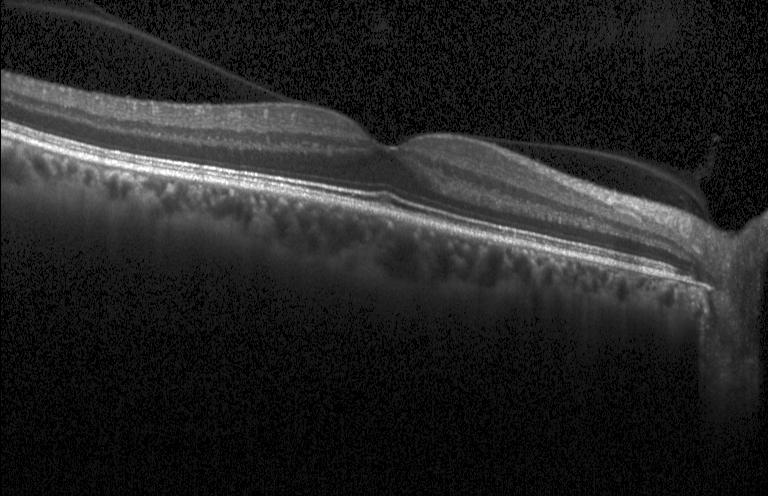

Retinal OCT cross-section. Impression: no choroidal neovascularization, diabetic macular edema, or drusen.